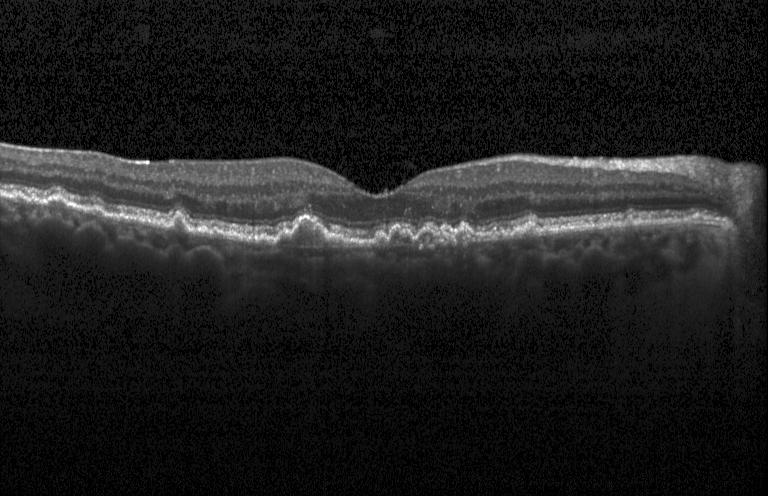
Heidelberg Spectralis OCT system. Horizontal scan through the fovea. OCT line scan — OCT finding: drusen.